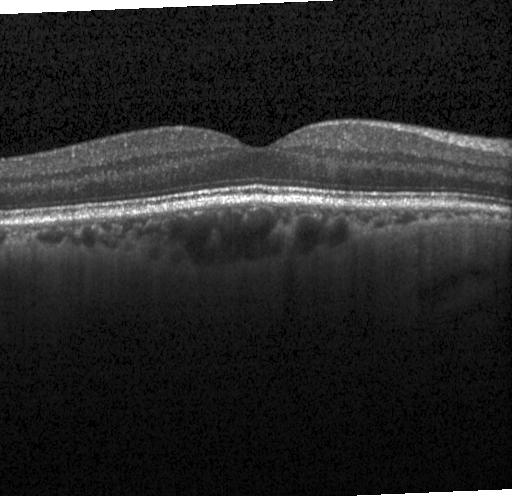

OCT line scan · horizontal scan through the fovea · spectral-domain OCT
Finding: no evidence of choroidal neovascularization, diabetic macular edema, or drusen.